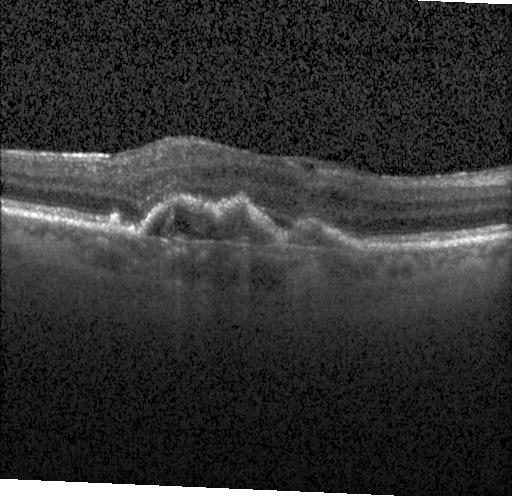 Optical coherence tomography scan
A choroidal neovascular membrane.